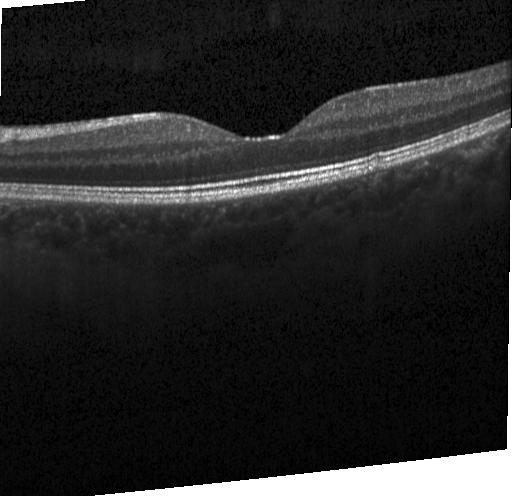 Assessment: no evidence of choroidal neovascularization, diabetic macular edema, or drusen.